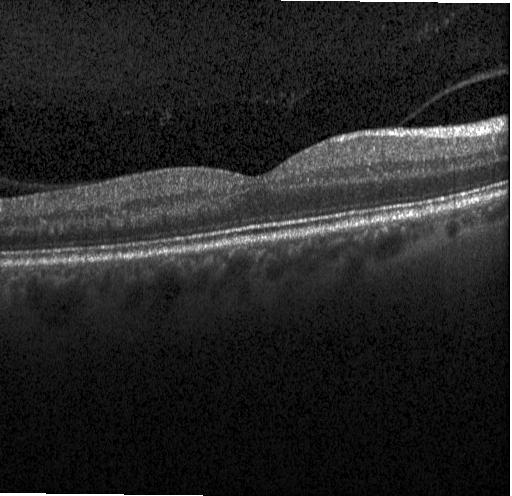 Retinal OCT cross-section, Heidelberg Spectralis OCT system, horizontal scan through the fovea — Diagnosis: no choroidal neovascularization, diabetic macular edema, or drusen.